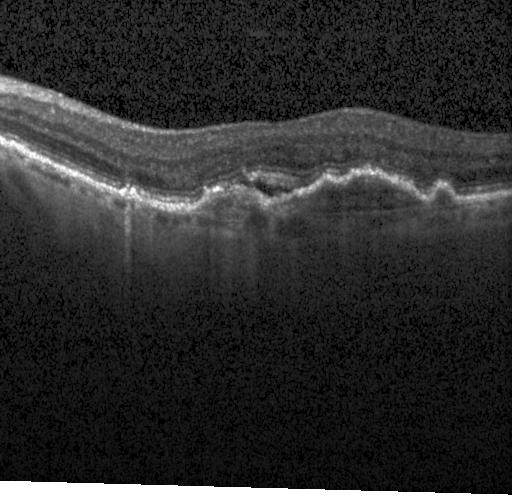

Macular scan · retinal OCT B-scan — Assessment: choroidal neovascularization.